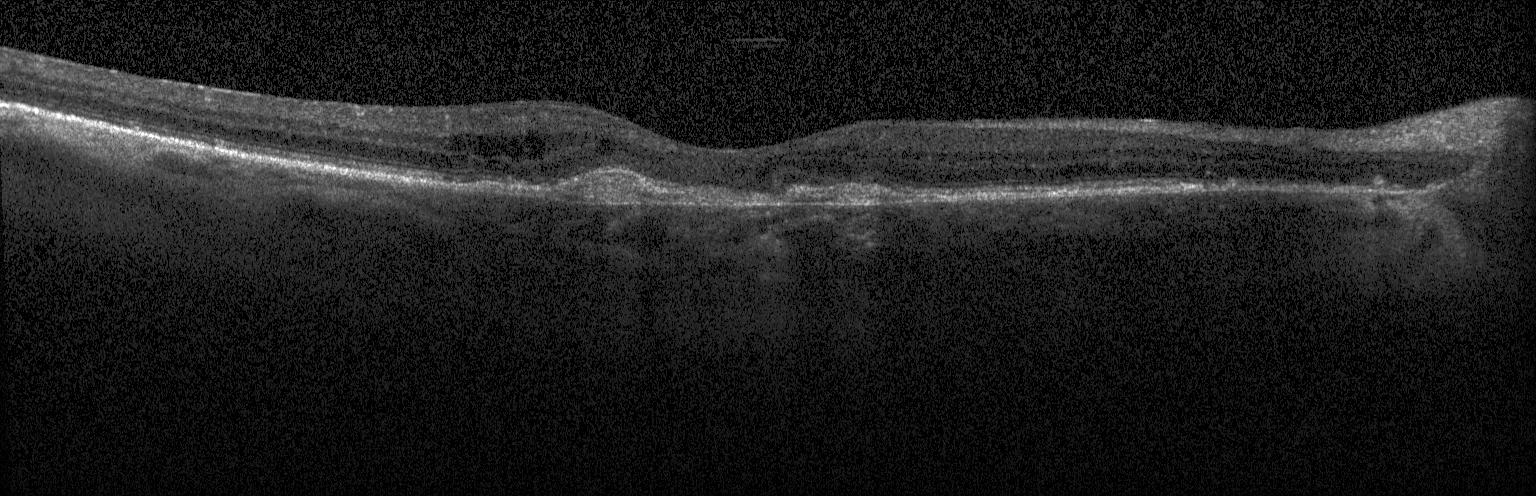
Spectral-domain OCT · retinal OCT cross-section
Impression: choroidal neovascularization (CNV).